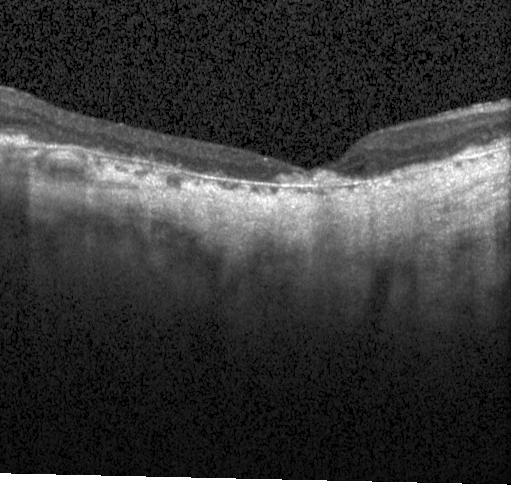
Optical coherence tomography B-scan · spectral-domain OCT · macular scan · Heidelberg Spectralis OCT system
This B-scan demonstrates a choroidal neovascular membrane.